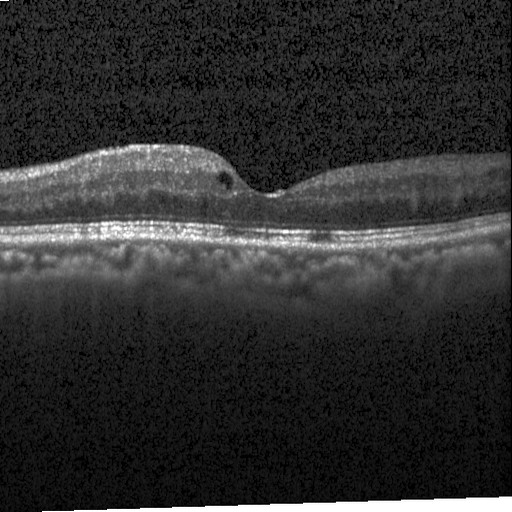 OCT B-scan. Finding: DME.